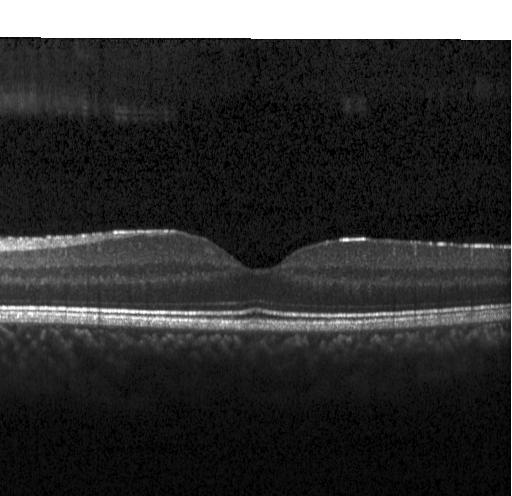
Spectral-domain OCT, optical coherence tomography B-scan, Heidelberg Spectralis OCT system
No evidence of choroidal neovascularization, diabetic macular edema, or drusen.